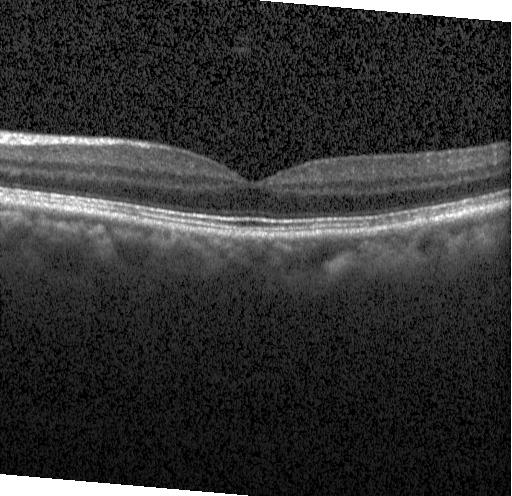

Finding: neither choroidal neovascularization, diabetic macular edema, nor drusen.